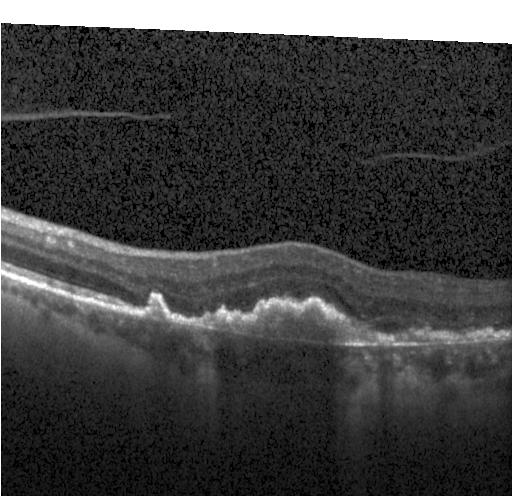

OCT B-scan showing choroidal neovascularization.